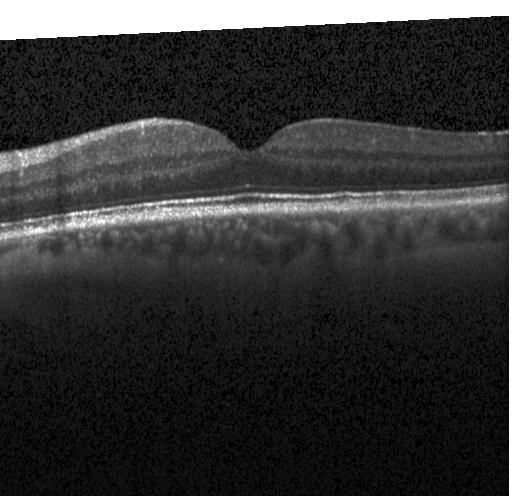 Spectral-domain optical coherence tomography, optical coherence tomography scan, macular scan — OCT finding: neither choroidal neovascularization, diabetic macular edema, nor drusen.